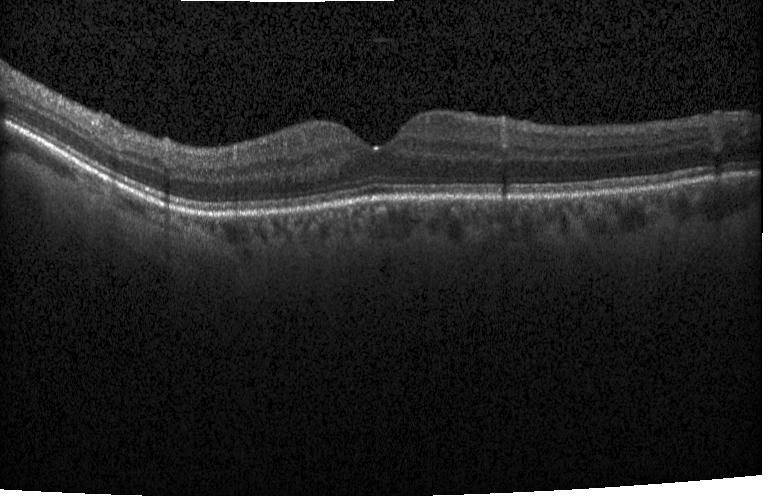

Impression: no CNV, DME, or drusen.